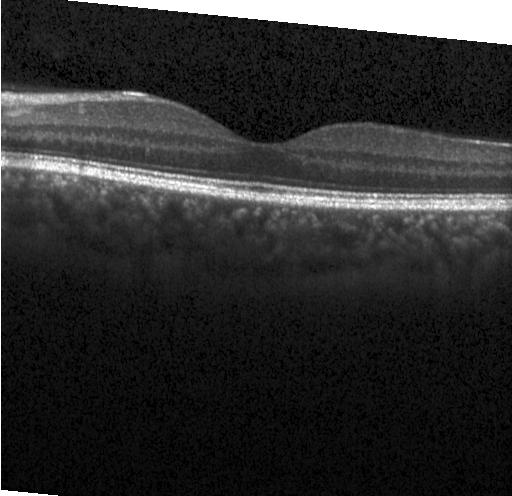 Centered on the fovea; retinal OCT B-scan. Diagnosis: neither choroidal neovascularization, diabetic macular edema, nor drusen.